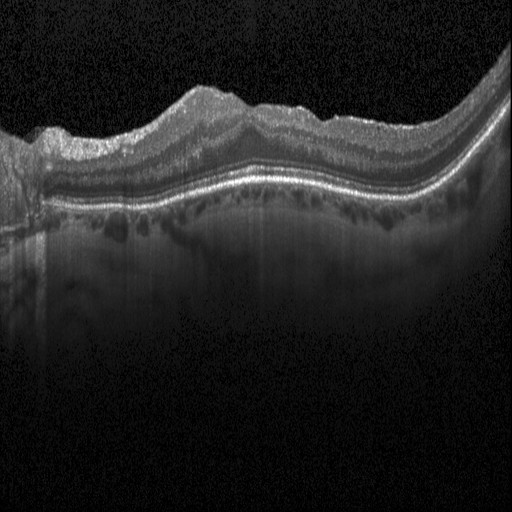 Macular OCT: diabetic macular edema.